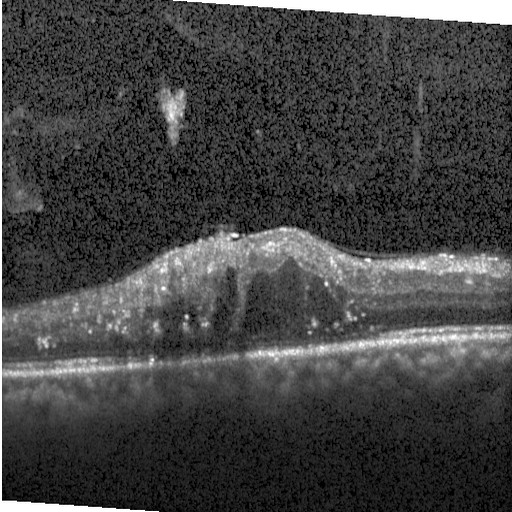 Diabetic macular edema (DME).